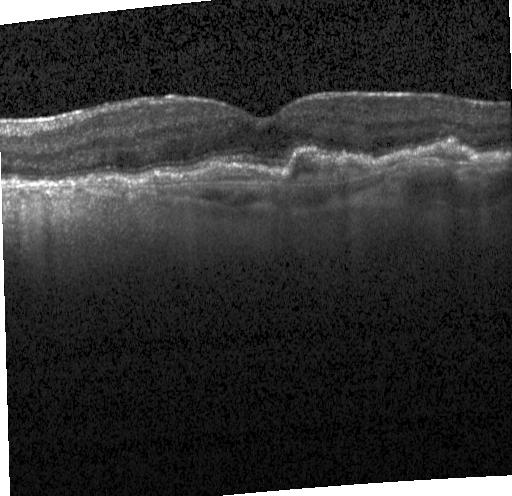 Spectral-domain OCT; optical coherence tomography B-scan.
Dx: a choroidal neovascular membrane.